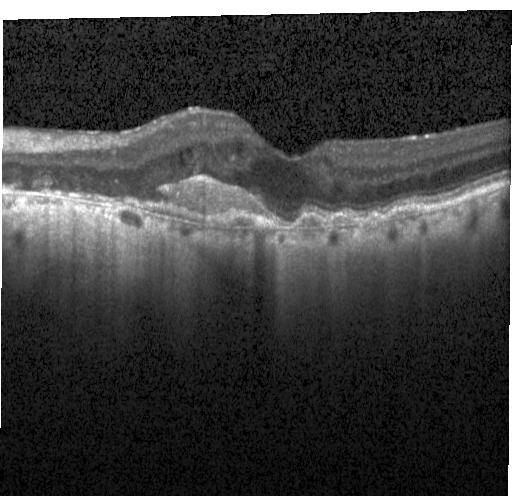 Instrument: Heidelberg Spectralis. Fovea-centered. Optical coherence tomography B-scan. Impression: CNV.